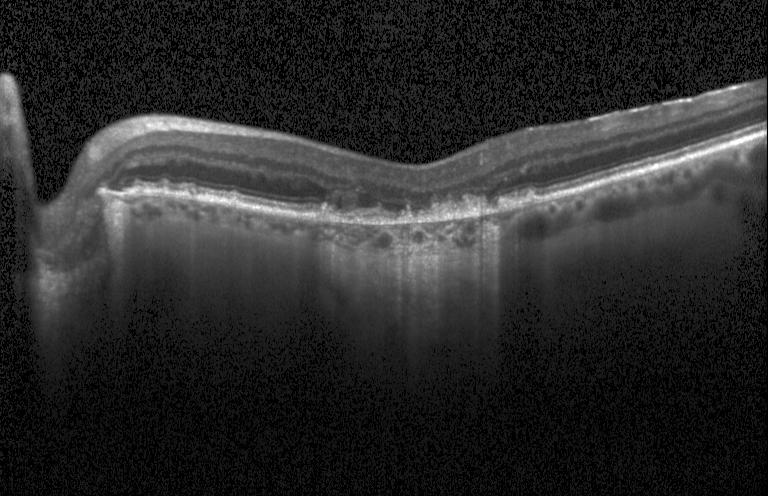

Optical coherence tomography B-scan. Macular scan
A choroidal neovascular membrane.